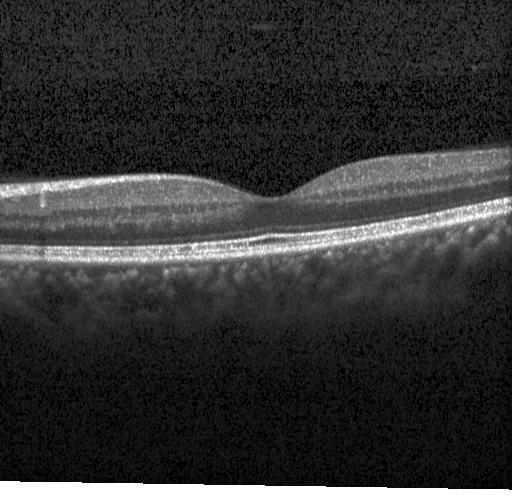 Retinal OCT B-scan, spectral-domain optical coherence tomography, fovea-centered — OCT finding: no choroidal neovascularization, diabetic macular edema, or drusen.